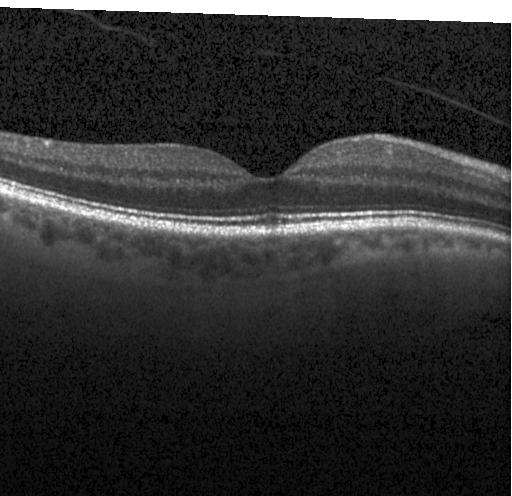
Dx: neither choroidal neovascularization, diabetic macular edema, nor drusen.